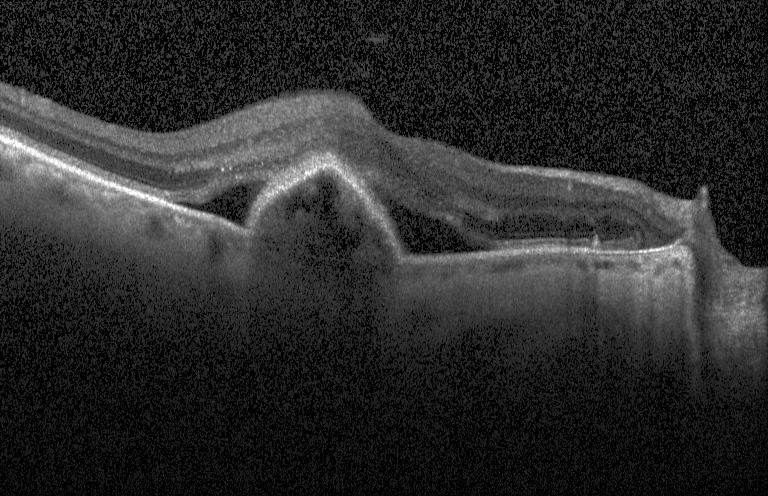 Impression: a choroidal neovascular membrane.